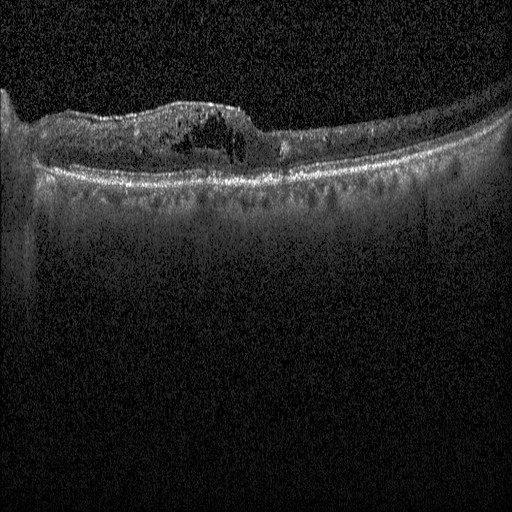
Retinal OCT B-scan, SD-OCT
Diagnosis: DME.